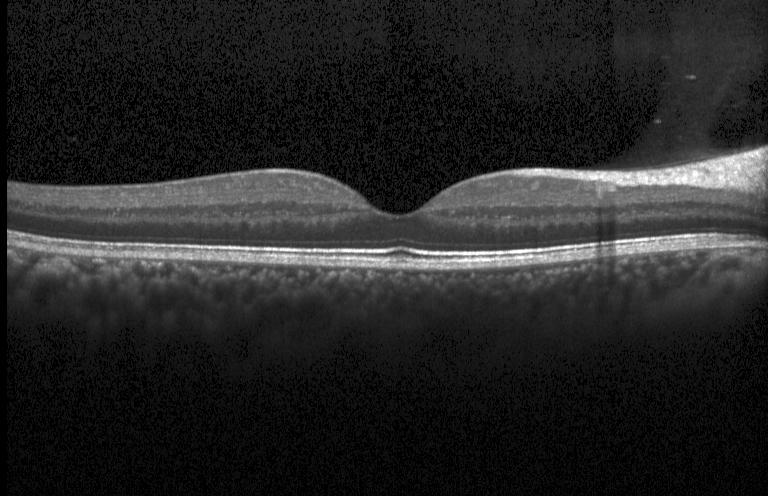

Impression: no choroidal neovascularization, diabetic macular edema, or drusen.